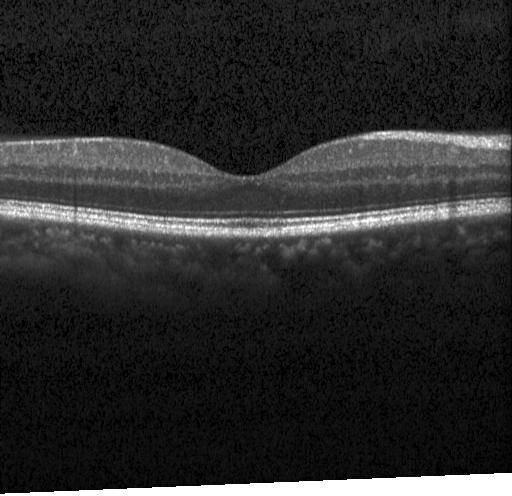 Optical coherence tomography B-scan — Finding: no CNV, no DME, and no drusen.